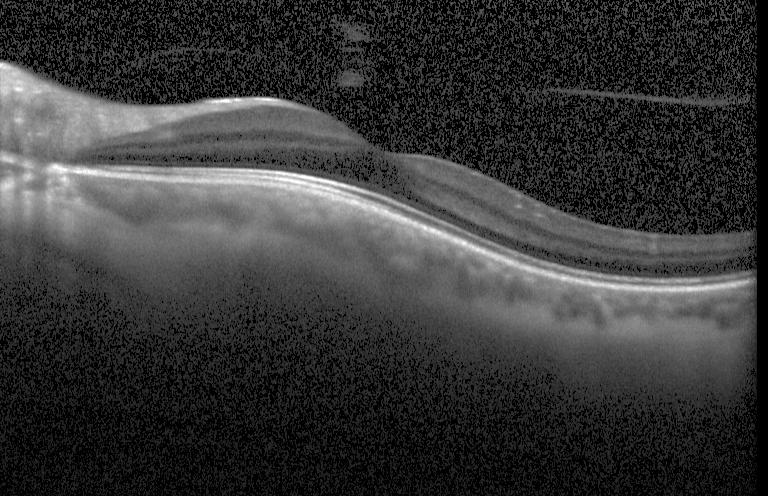

Optical coherence tomography scan.
Impression: no CNV, no DME, and no drusen.